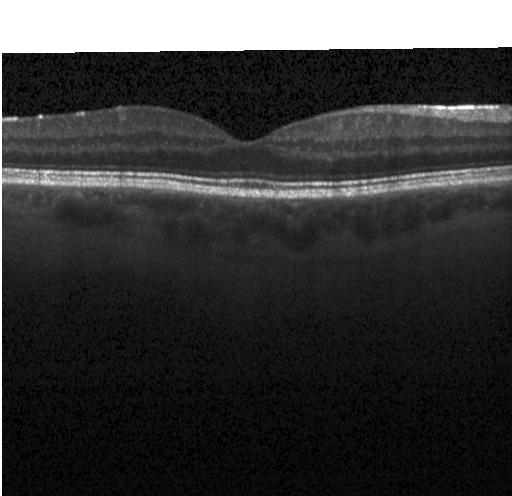 Retinal OCT cross-section showing no choroidal neovascularization, no diabetic macular edema, and no drusen.